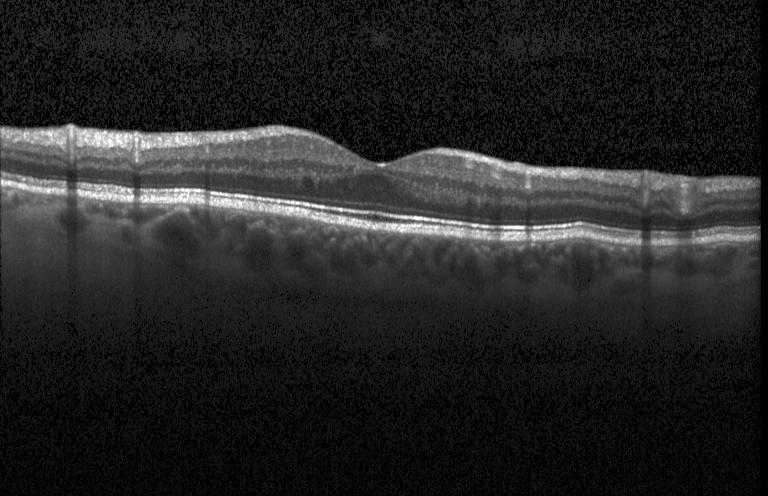

OCT line scan
Neither choroidal neovascularization, diabetic macular edema, nor drusen.